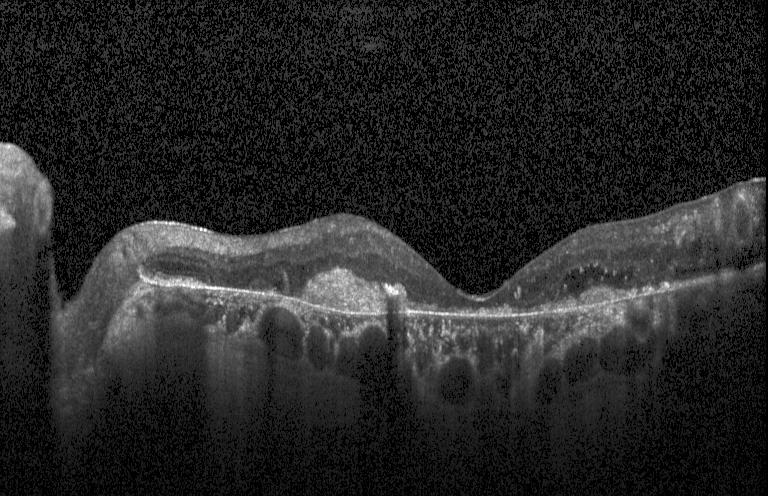
Optical coherence tomography scan · Heidelberg Spectralis OCT system — Assessment: choroidal neovascularization (CNV).